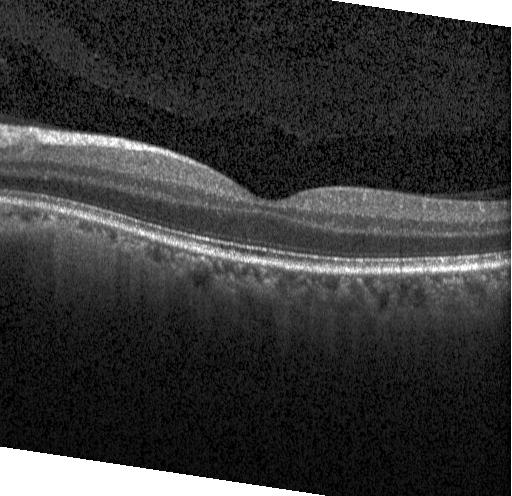
OCT finding: neither choroidal neovascularization, diabetic macular edema, nor drusen.